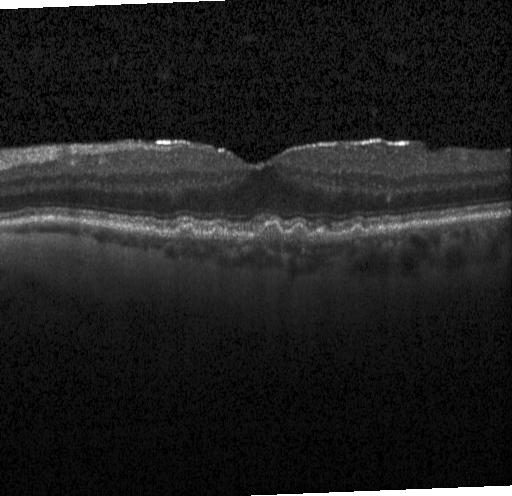 Heidelberg Spectralis OCT system. Spectral-domain OCT. OCT line scan
Finding: drusen.